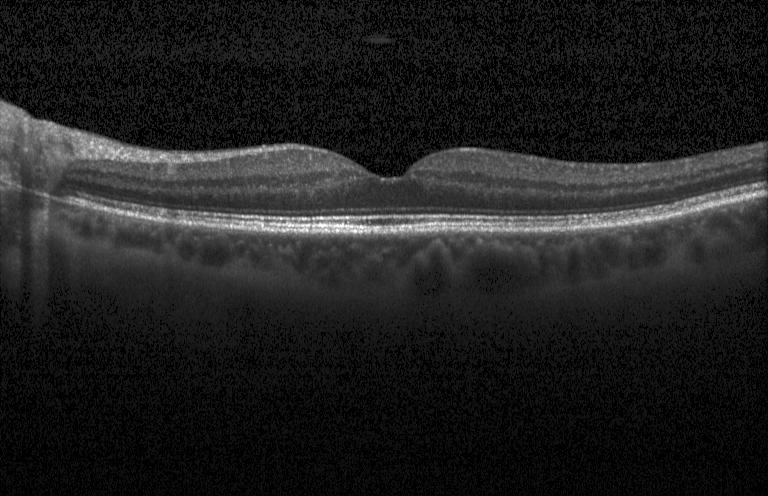
This B-scan demonstrates no evidence of choroidal neovascularization, diabetic macular edema, or drusen.